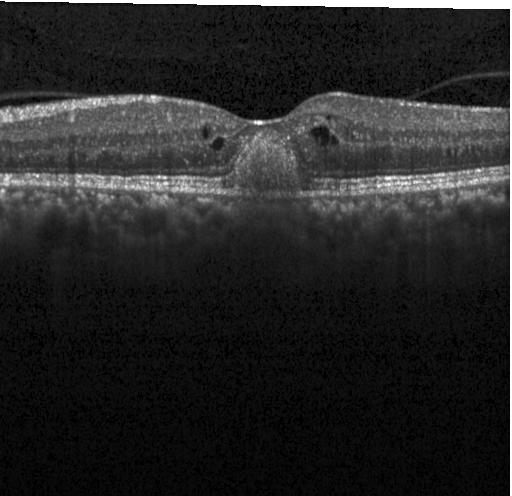 OCT B-scan.
Finding: choroidal neovascularization (CNV).